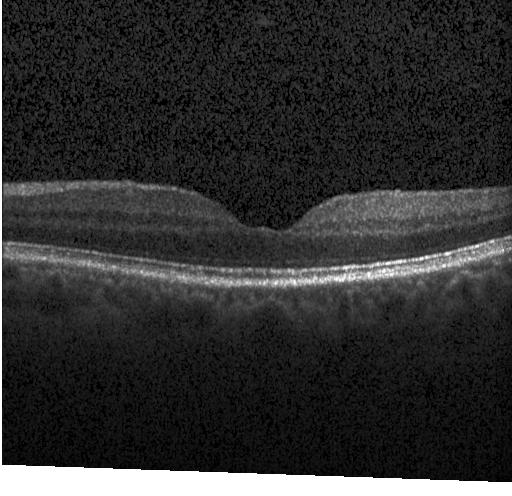
Spectral-domain OCT B-scan: neither choroidal neovascularization, diabetic macular edema, nor drusen.